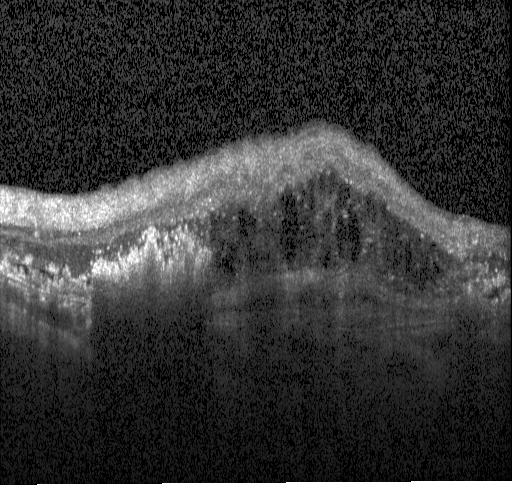
OCT line scan · centered on the fovea
Finding: DME.